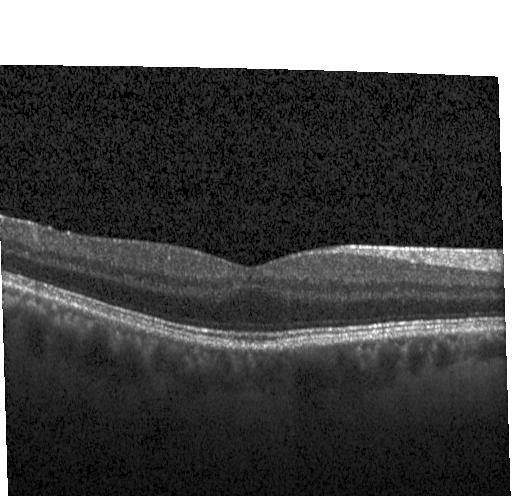

The scan shows neither choroidal neovascularization, diabetic macular edema, nor drusen.